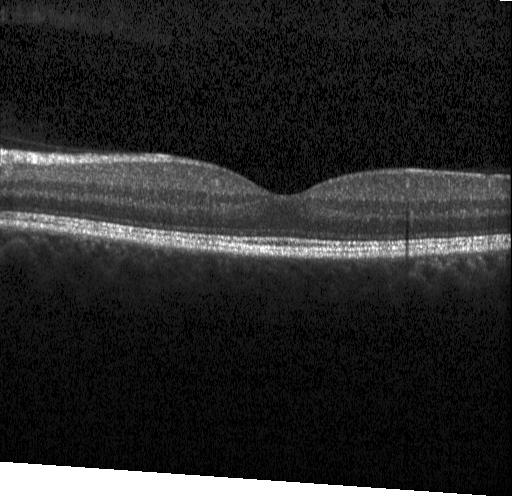

Retinal OCT cross-section. Diagnosis: no choroidal neovascularization, no diabetic macular edema, and no drusen.